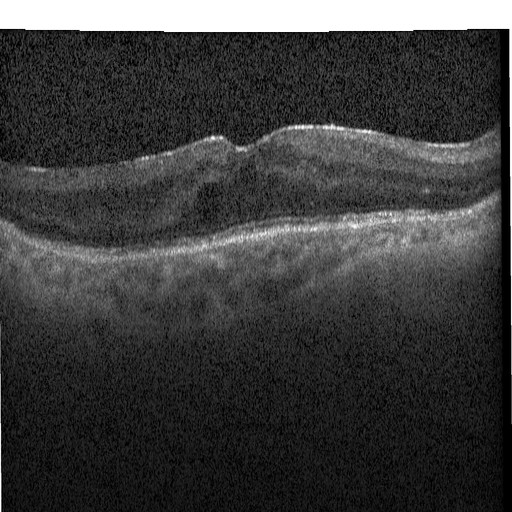 Fovea-centered; optical coherence tomography B-scan
Macular OCT: diabetic macular edema (DME).